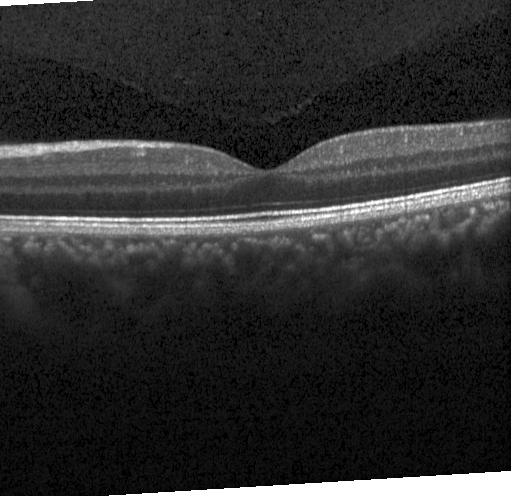 Heidelberg Spectralis. OCT B-scan. Macular scan. Spectral-domain optical coherence tomography.
Dx: no choroidal neovascularization, diabetic macular edema, or drusen.